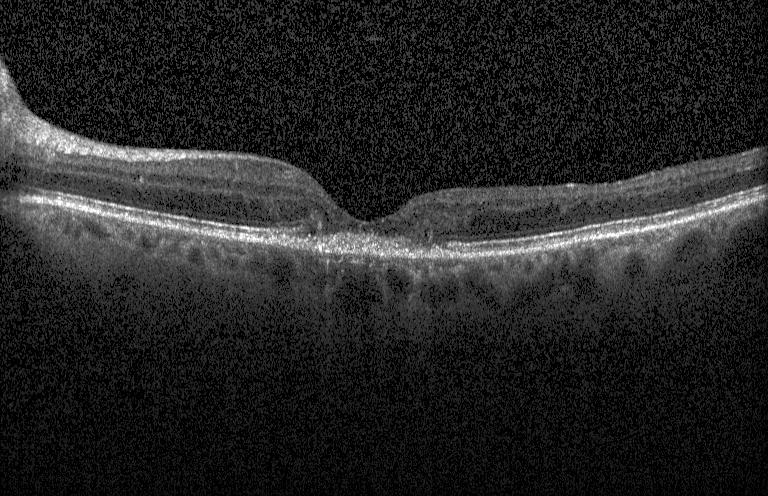 OCT line scan, SD-OCT
Impression: a choroidal neovascular membrane.